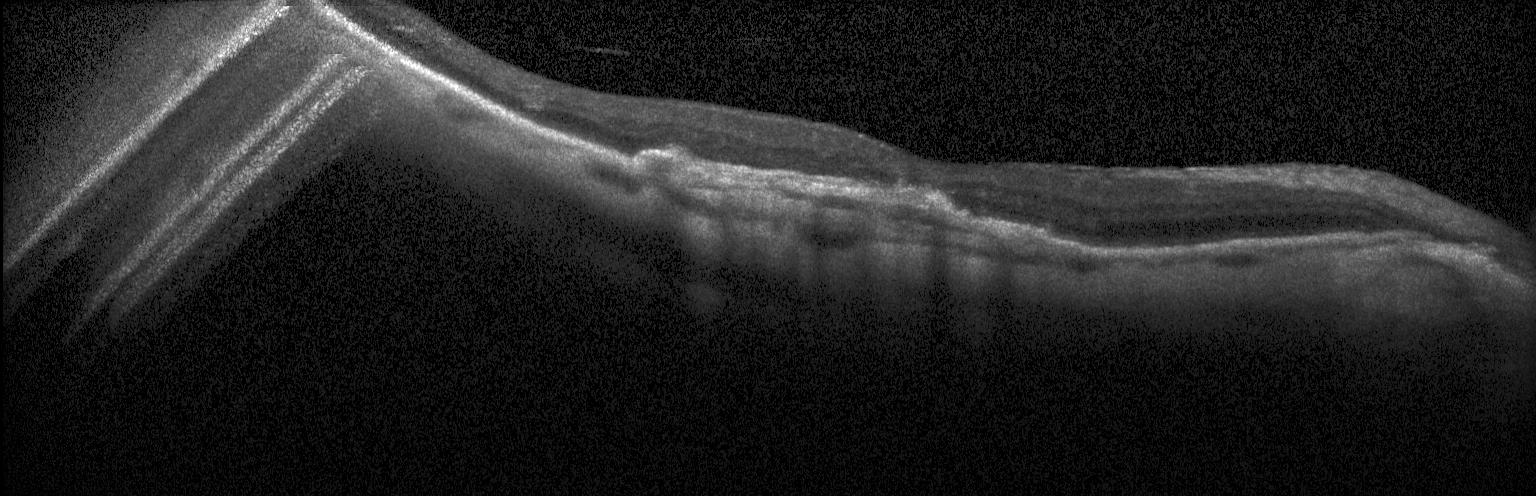

Retinal OCT cross-section — Macular OCT: a choroidal neovascular membrane.